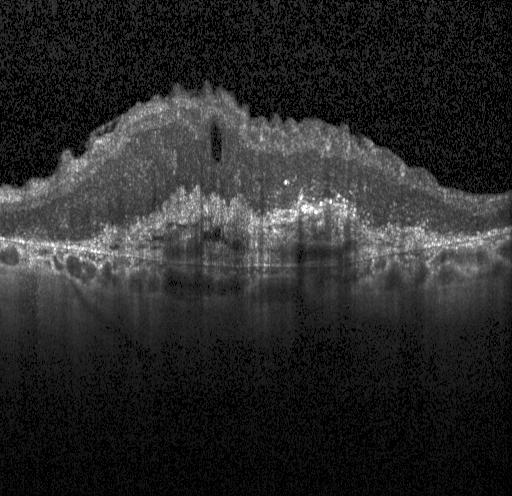

Impression: choroidal neovascularization (CNV).